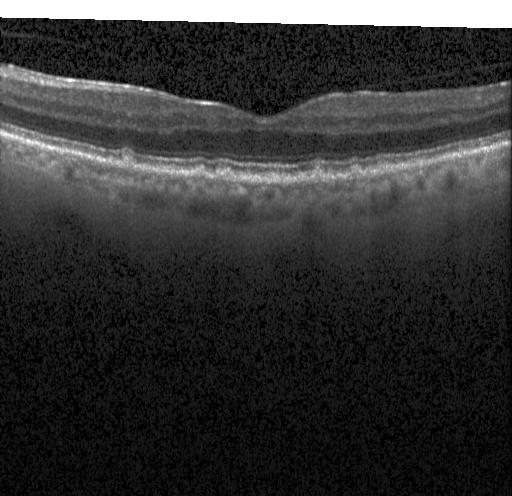 Impression: multiple drusen.